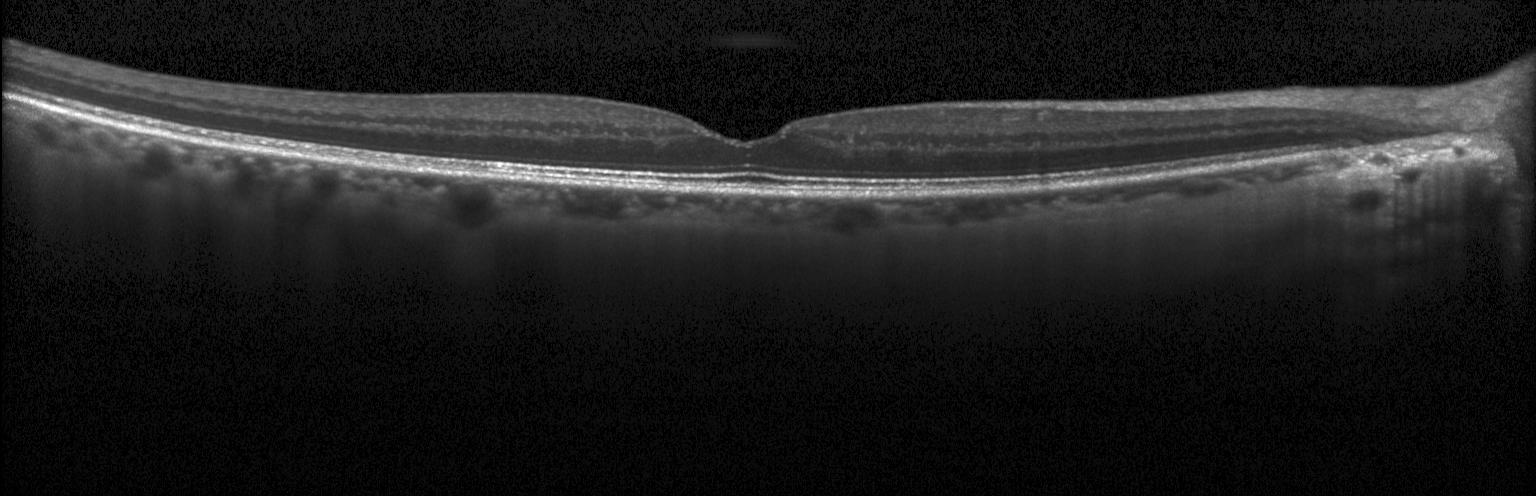
Retinal OCT cross-section showing no choroidal neovascularization, diabetic macular edema, or drusen.